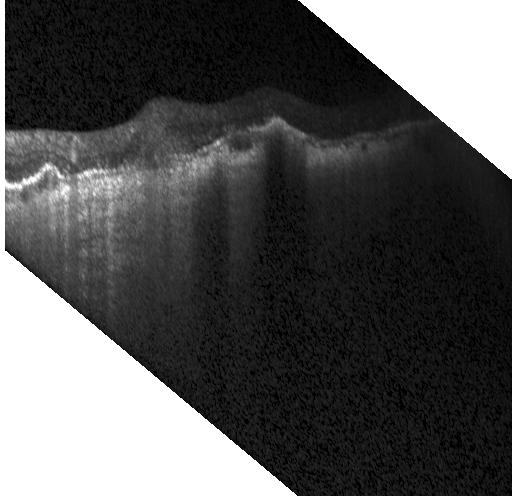

SD-OCT · OCT B-scan · fovea-centered · Heidelberg Spectralis OCT system.
Impression: a choroidal neovascular membrane.